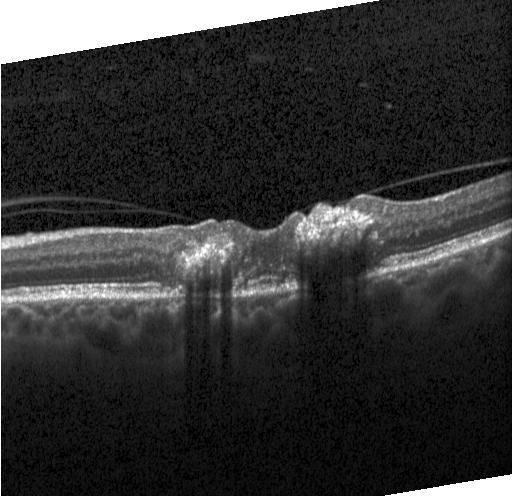 Fovea-centered. Optical coherence tomography scan. SD-OCT. Heidelberg Spectralis OCT system
Macular OCT: choroidal neovascularization (CNV).